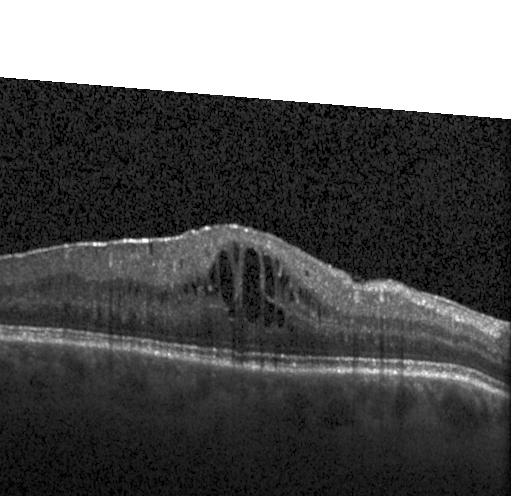
OCT line scan · SD-OCT · Heidelberg Spectralis OCT system · horizontal scan through the fovea. Finding: DME.